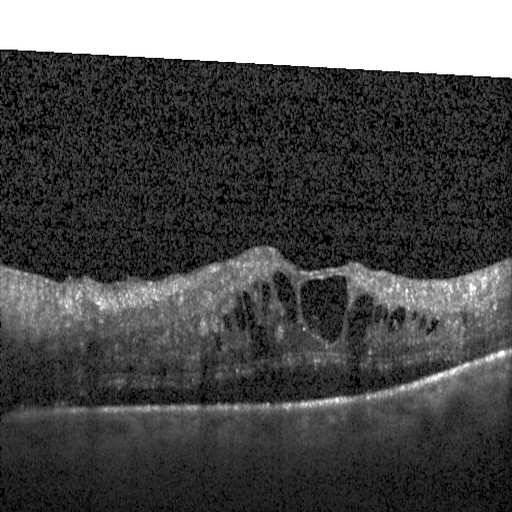 Retinal OCT cross-section · spectral-domain OCT · Heidelberg Spectralis OCT system
Impression: DME.